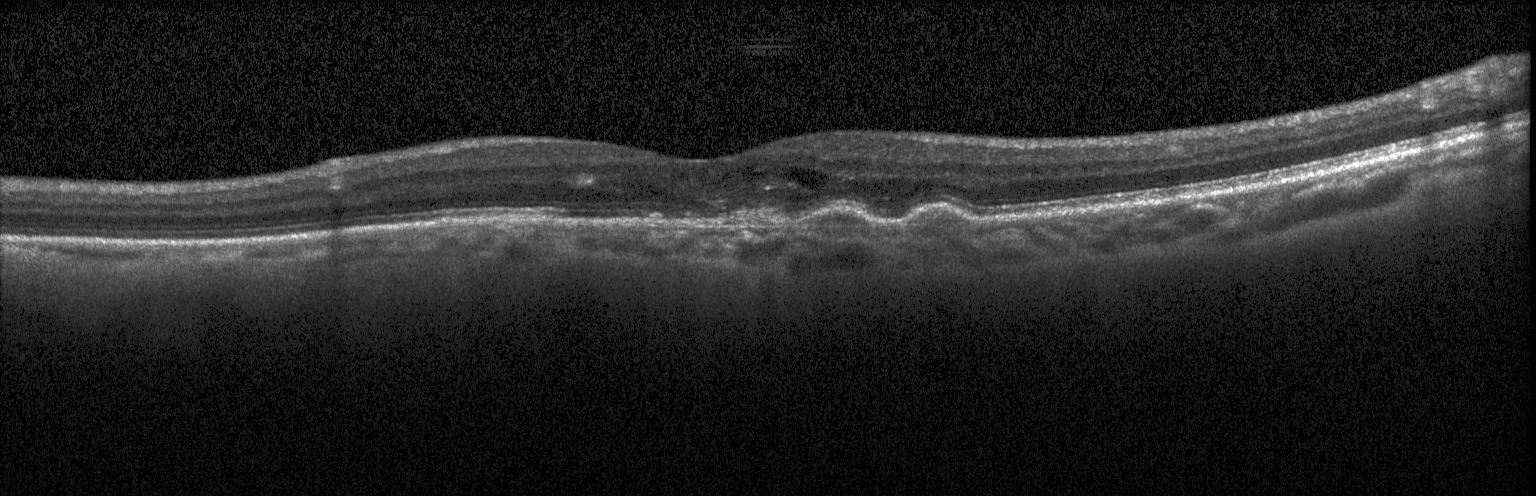 Optical coherence tomography B-scan — Diagnosis: choroidal neovascularization.